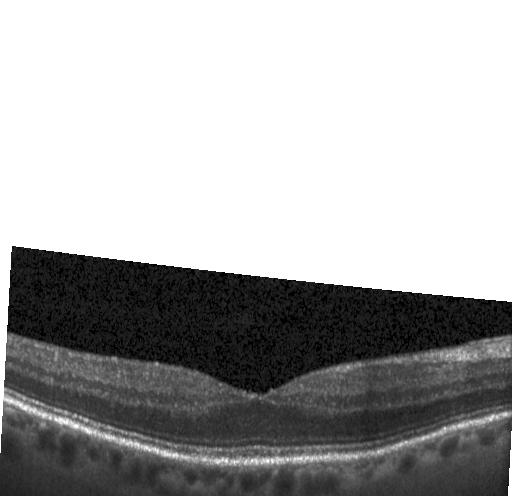
Spectral-domain OCT · OCT line scan · through the macula · acquired on a Heidelberg Spectralis. OCT finding: no evidence of choroidal neovascularization, diabetic macular edema, or drusen.